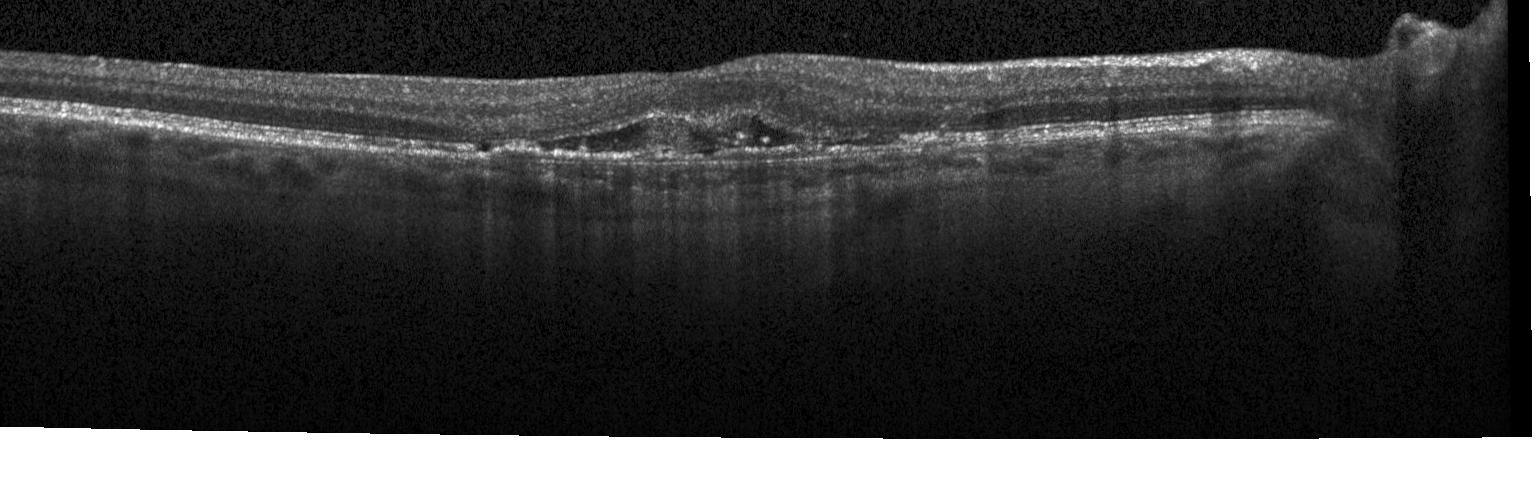
OCT finding: a choroidal neovascular membrane.